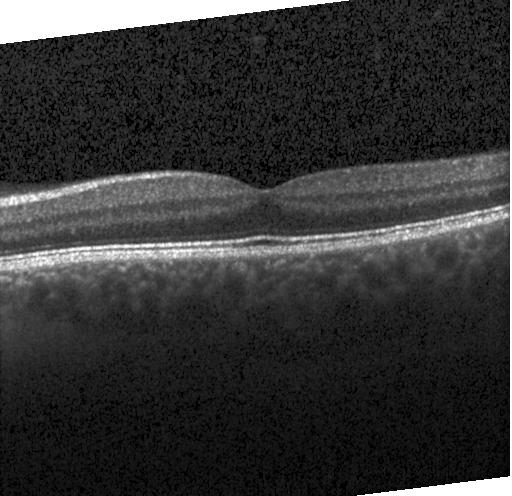
OCT scan showing no CNV, no DME, and no drusen.